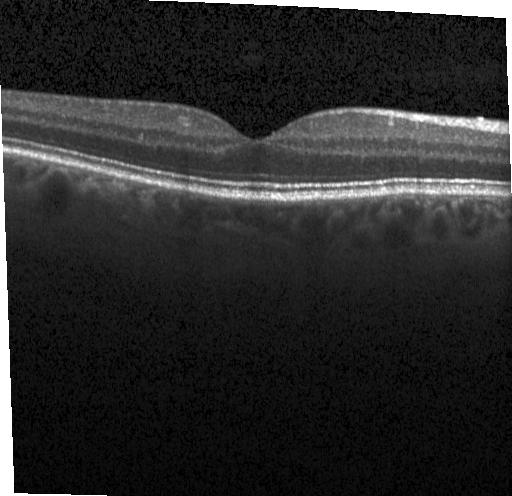
Optical coherence tomography scan · through the macula · Heidelberg Spectralis.
Finding: no choroidal neovascularization, diabetic macular edema, or drusen.